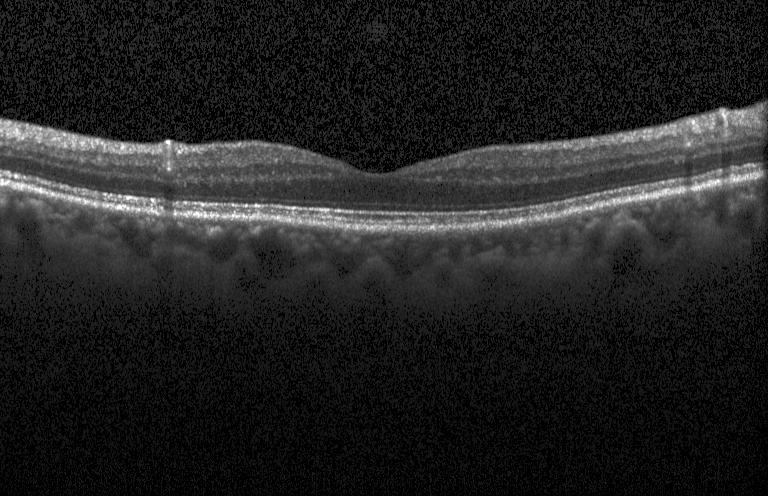

Retinal OCT B-scan, Heidelberg Spectralis.
Diagnosis: neither CNV, DME, nor drusen.